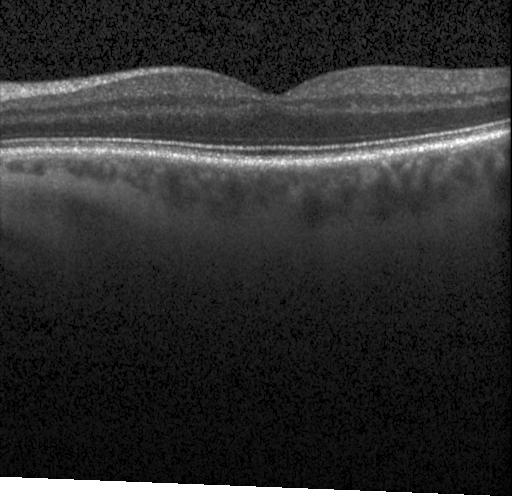
Diagnosis: no choroidal neovascularization, diabetic macular edema, or drusen.